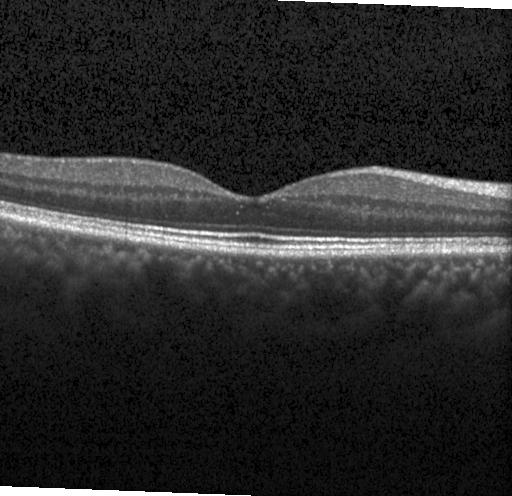

Assessment: no choroidal neovascularization, diabetic macular edema, or drusen.